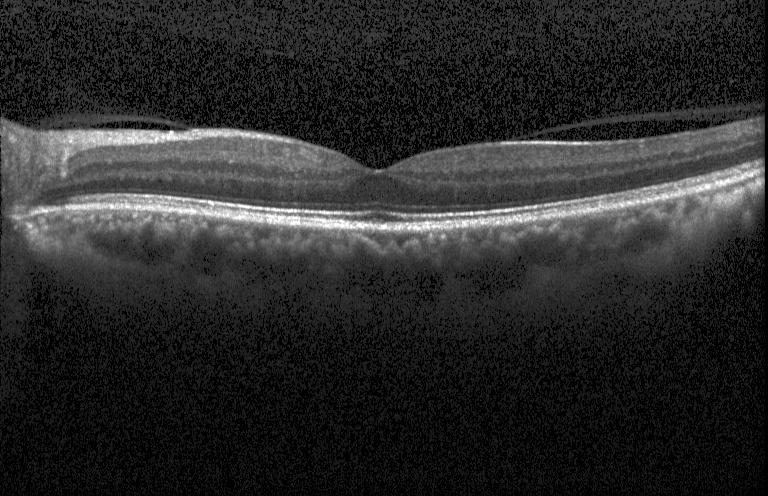 Retinal OCT cross-section · acquired on a Heidelberg Spectralis · through the macula · spectral-domain optical coherence tomography. Impression: no choroidal neovascularization, diabetic macular edema, or drusen.